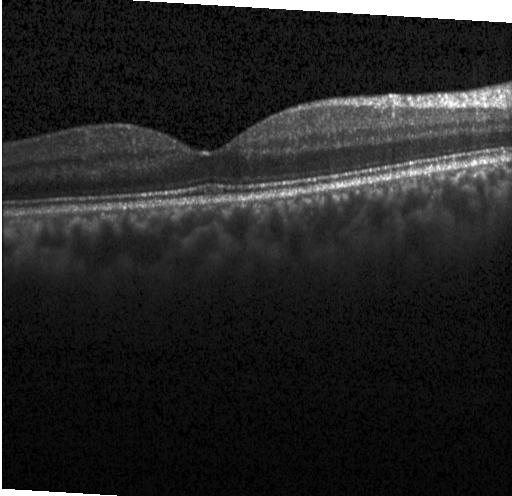 Retinal OCT B-scan; spectral-domain OCT; instrument: Heidelberg Spectralis. Neither CNV, DME, nor drusen.